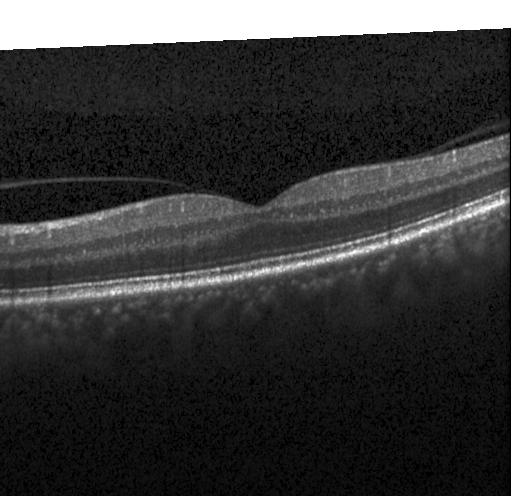

Finding: no evidence of CNV, DME, or drusen.